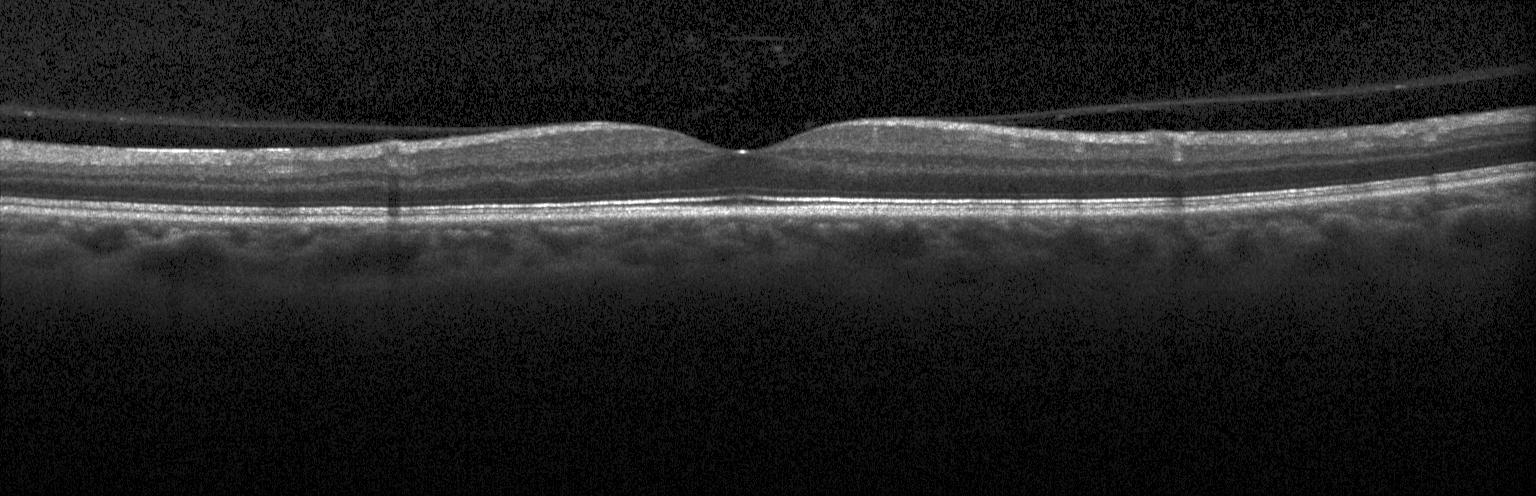 Instrument: Heidelberg Spectralis, through the macula, OCT line scan
Impression: no evidence of choroidal neovascularization, diabetic macular edema, or drusen.